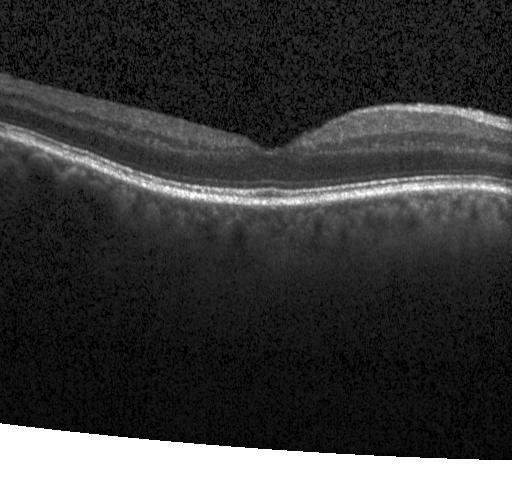 Optical coherence tomography B-scan. Horizontal scan through the fovea. Macular OCT: neither choroidal neovascularization, diabetic macular edema, nor drusen.